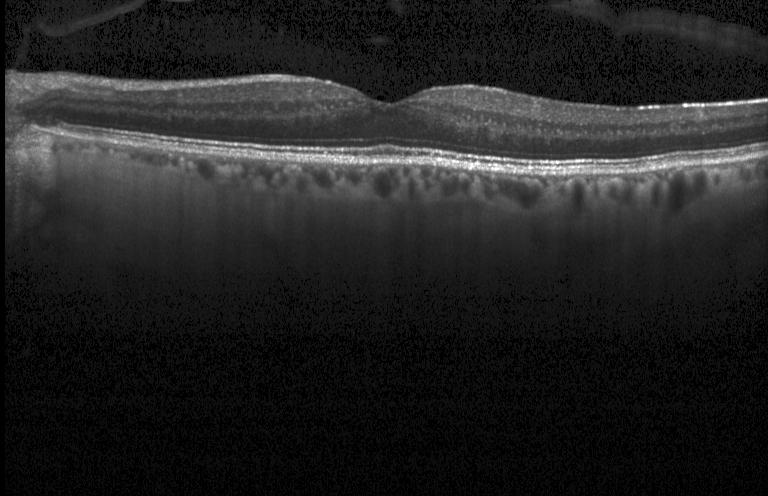 OCT line scan. The scan shows neither CNV, DME, nor drusen.